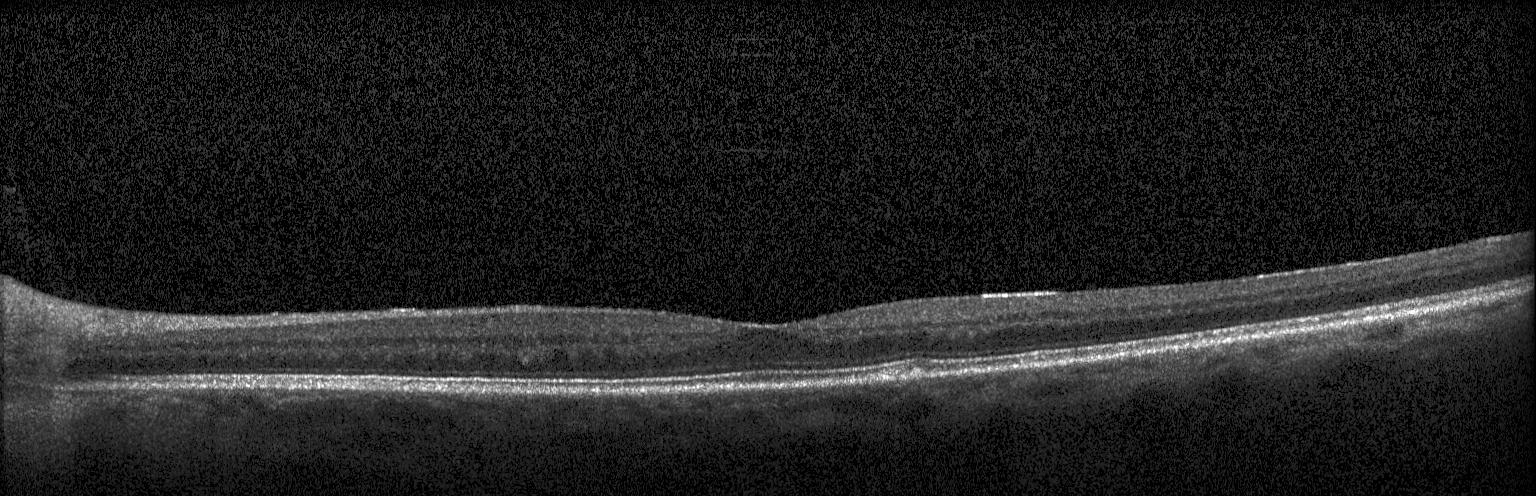

Assessment: no choroidal neovascularization, diabetic macular edema, or drusen.